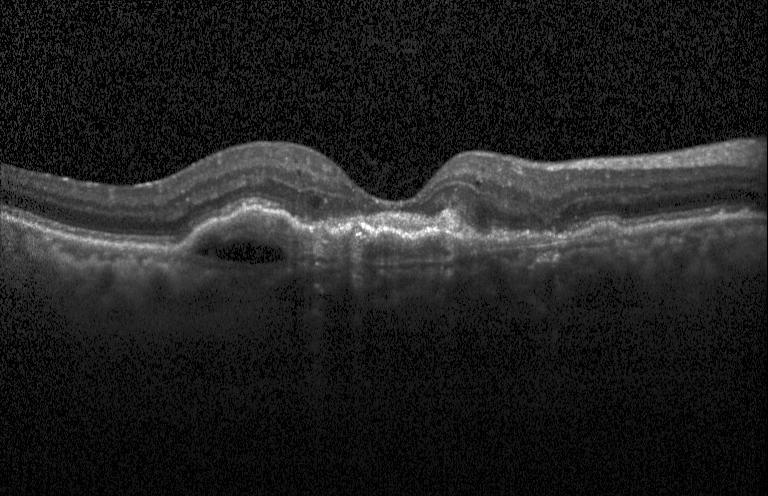

Optical coherence tomography B-scan
Diagnosis: a choroidal neovascular membrane.